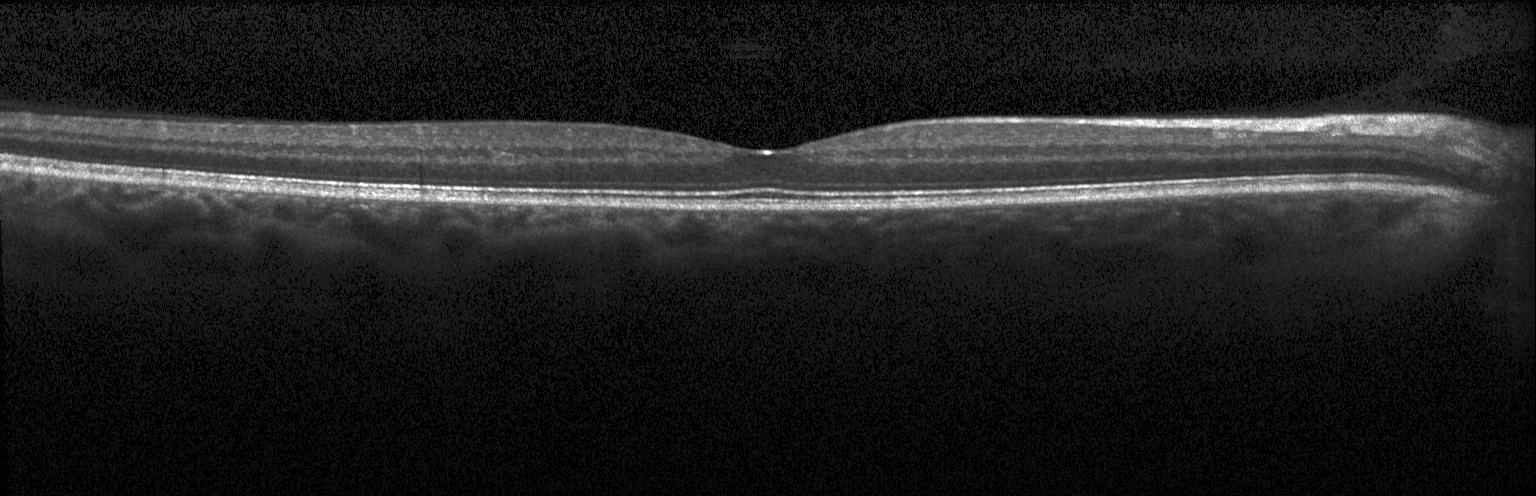 Heidelberg Spectralis OCT system; optical coherence tomography B-scan; SD-OCT. Diagnosis: no evidence of choroidal neovascularization, diabetic macular edema, or drusen.